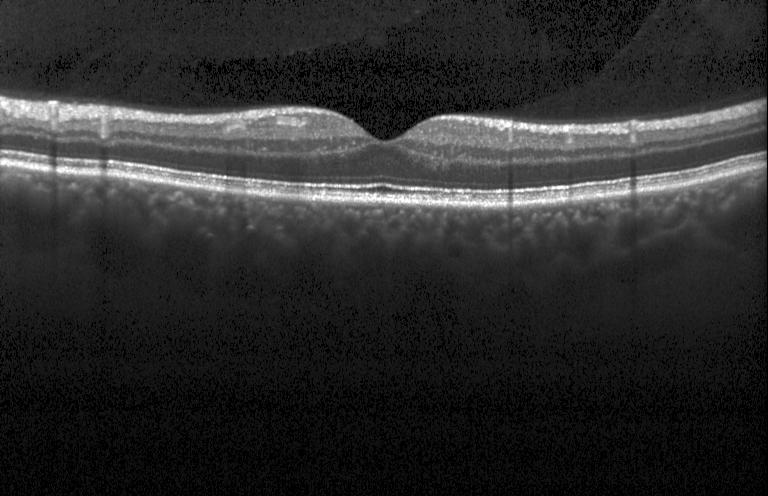
Diagnosis: neither CNV, DME, nor drusen.